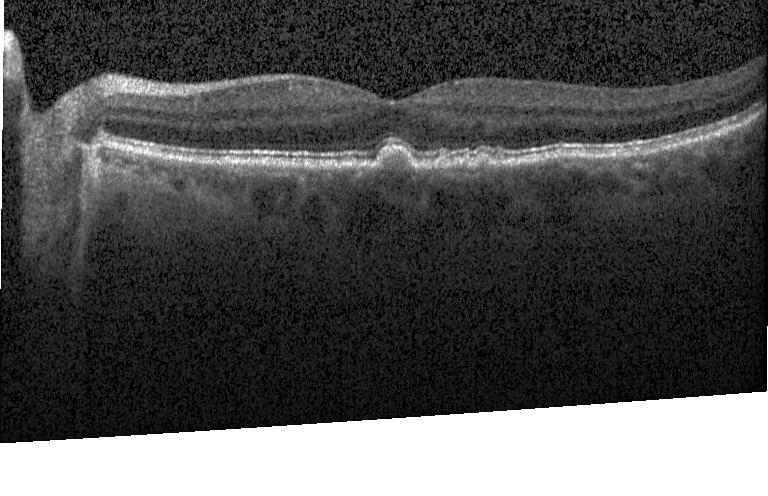
The scan shows multiple drusen.